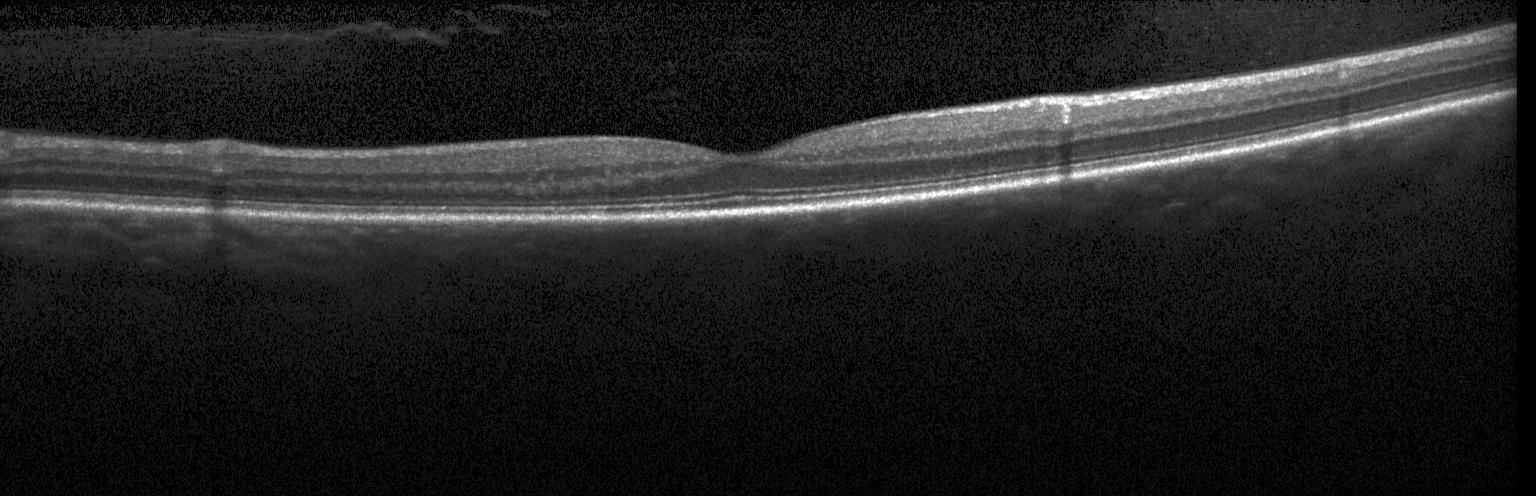
Spectral-domain OCT. Acquired on a Heidelberg Spectralis. Through the macula. Retinal OCT B-scan. Finding: no choroidal neovascularization, no diabetic macular edema, and no drusen.